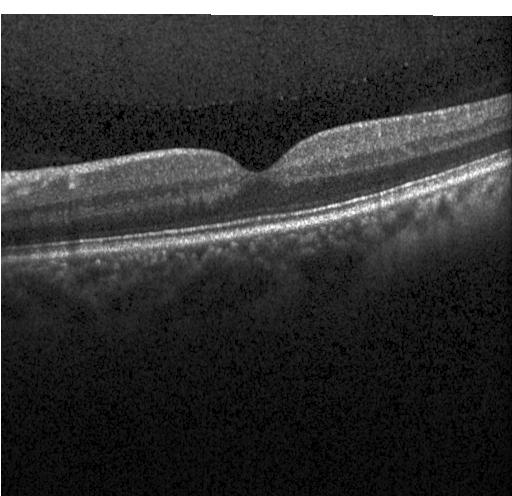
Optical coherence tomography scan — Impression: neither choroidal neovascularization, diabetic macular edema, nor drusen.